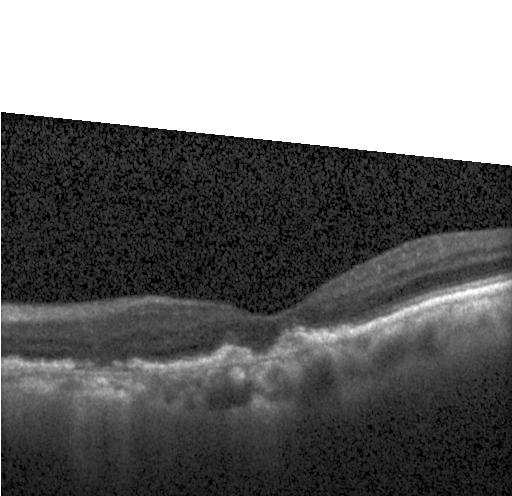 The scan shows a choroidal neovascular membrane.